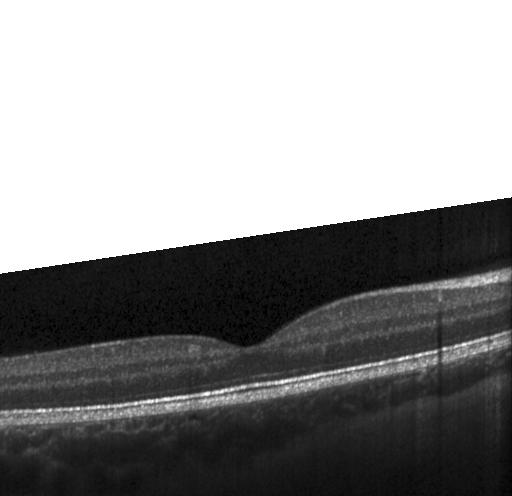 OCT scan showing neither choroidal neovascularization, diabetic macular edema, nor drusen.